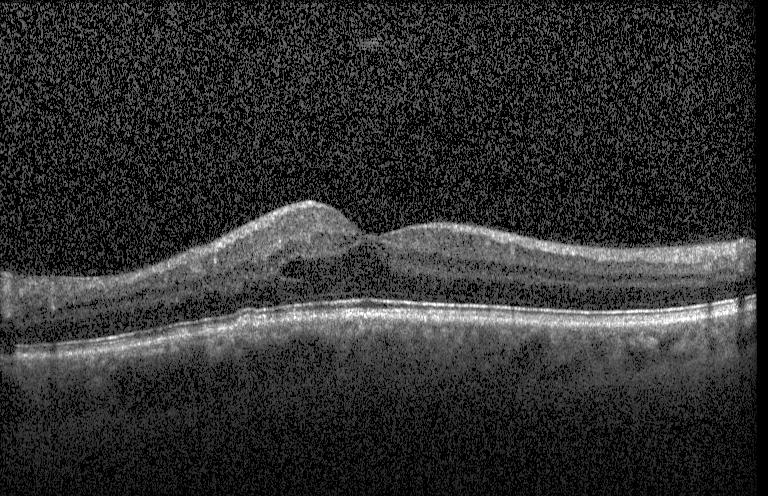
Spectral-domain optical coherence tomography · retinal OCT B-scan. Finding: DME.